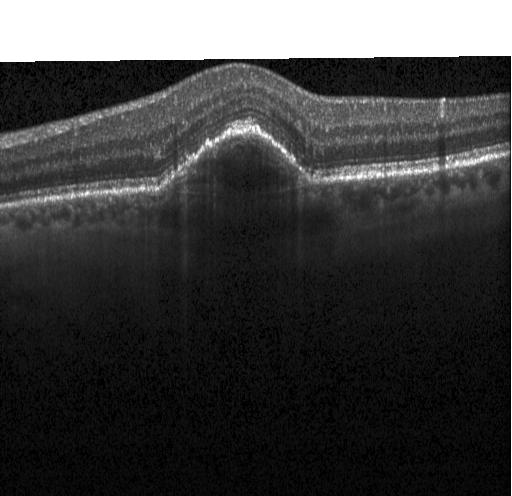
Optical coherence tomography B-scan.
Macular OCT: choroidal neovascularization (CNV).